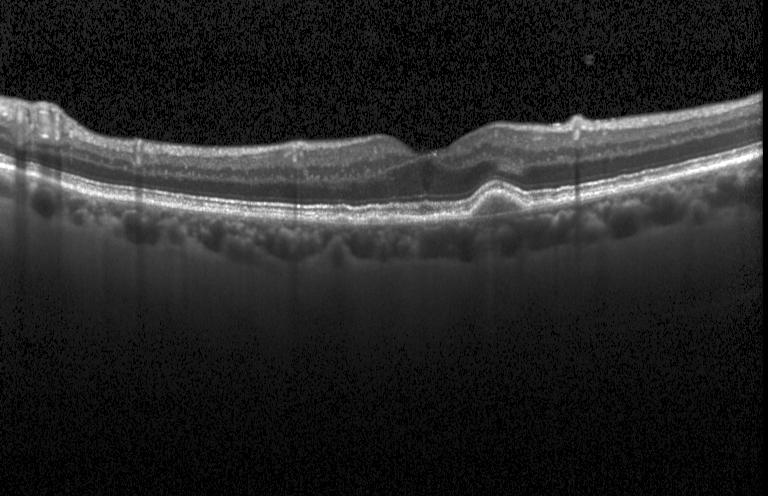 The scan shows multiple drusen.